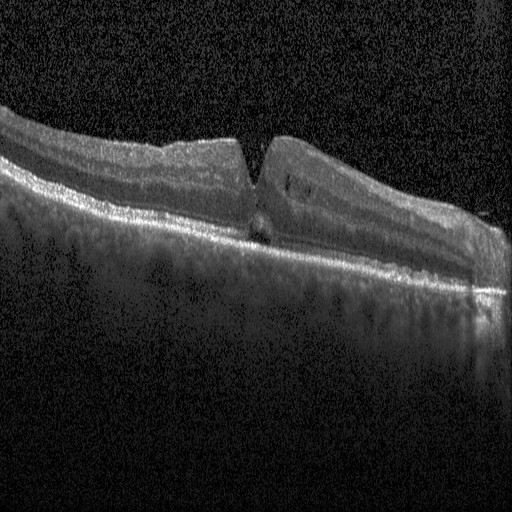
OCT B-scan · centered on the fovea.
Diagnosis: diabetic macular edema (DME).